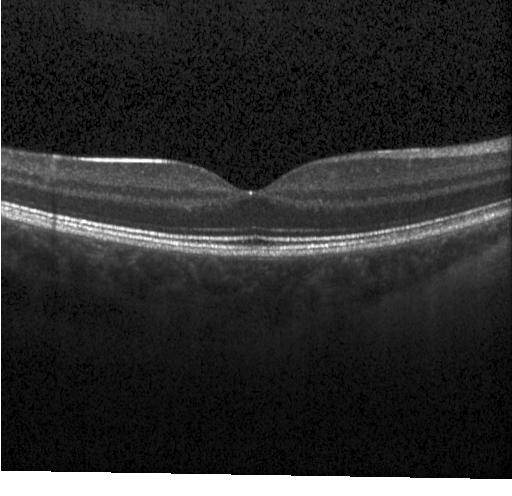

Through the macula · spectral-domain optical coherence tomography · OCT B-scan — Macular OCT: neither CNV, DME, nor drusen.